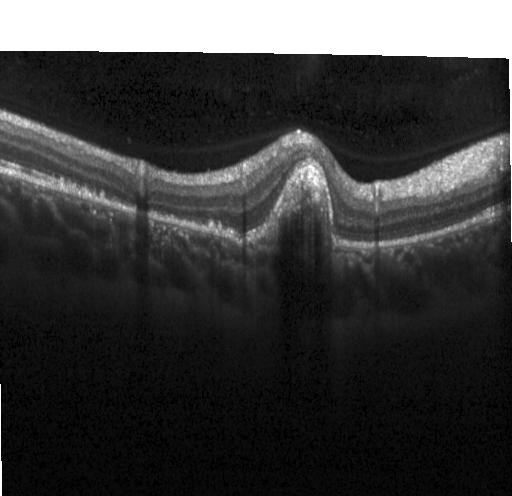

Optical coherence tomography scan. Through the macula. Acquired on a Heidelberg Spectralis. SD-OCT — Macular OCT: choroidal neovascularization.